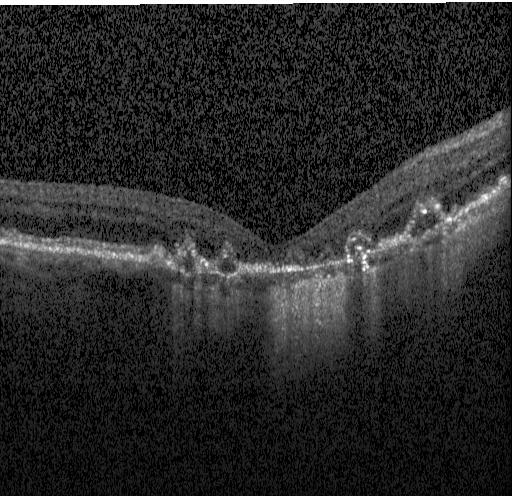
Macular OCT: a choroidal neovascular membrane.